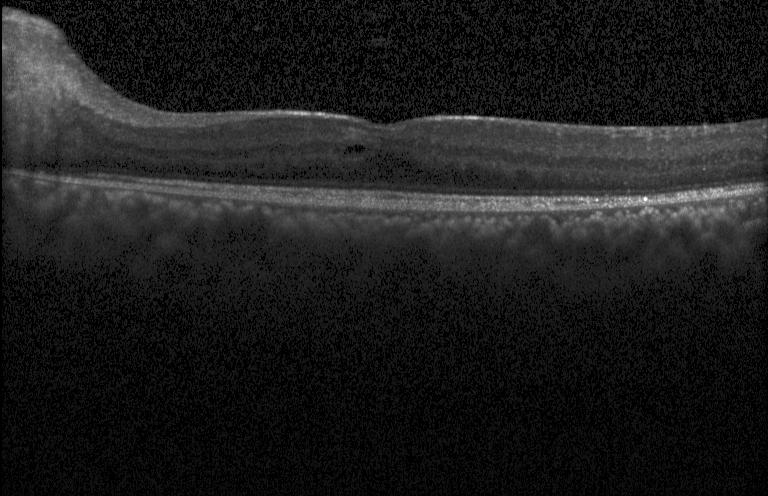
Diagnosis: diabetic macular edema.